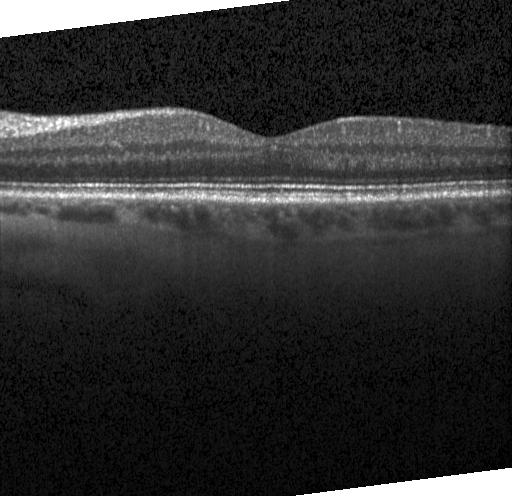
SD-OCT; Heidelberg Spectralis; OCT line scan.
Finding: neither CNV, DME, nor drusen.